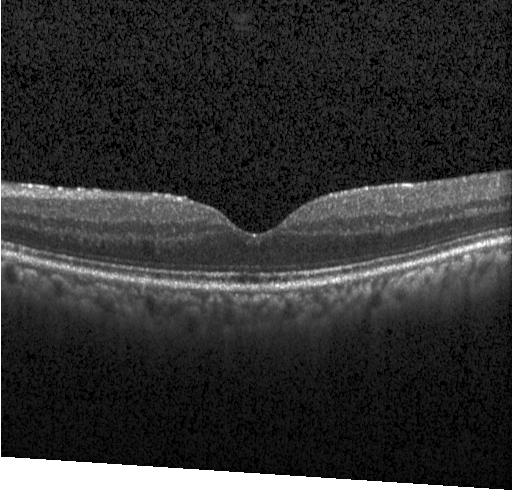
Macular OCT: no choroidal neovascularization, no diabetic macular edema, and no drusen.